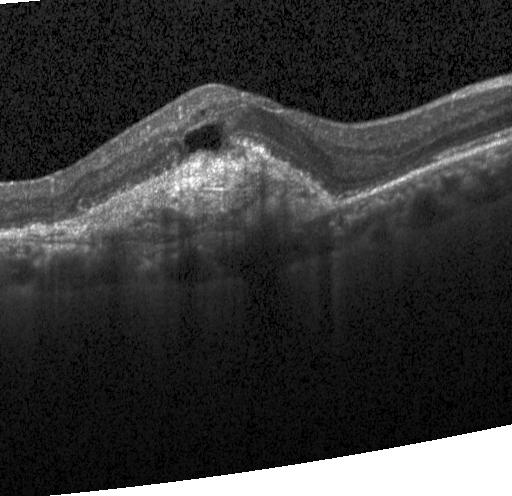
Retinal OCT cross-section, acquired on a Heidelberg Spectralis, SD-OCT. Impression: a choroidal neovascular membrane.